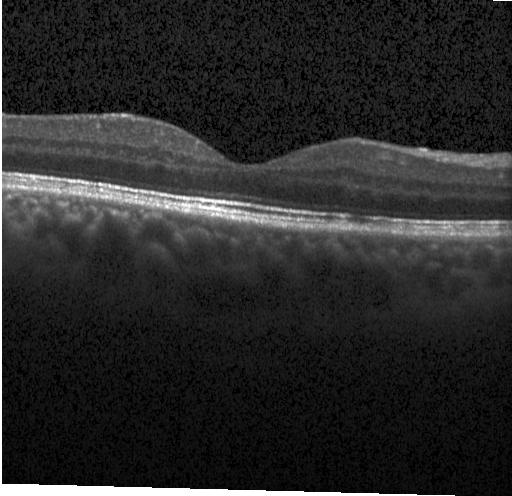
Retinal OCT B-scan. Macular OCT: no evidence of CNV, DME, or drusen.